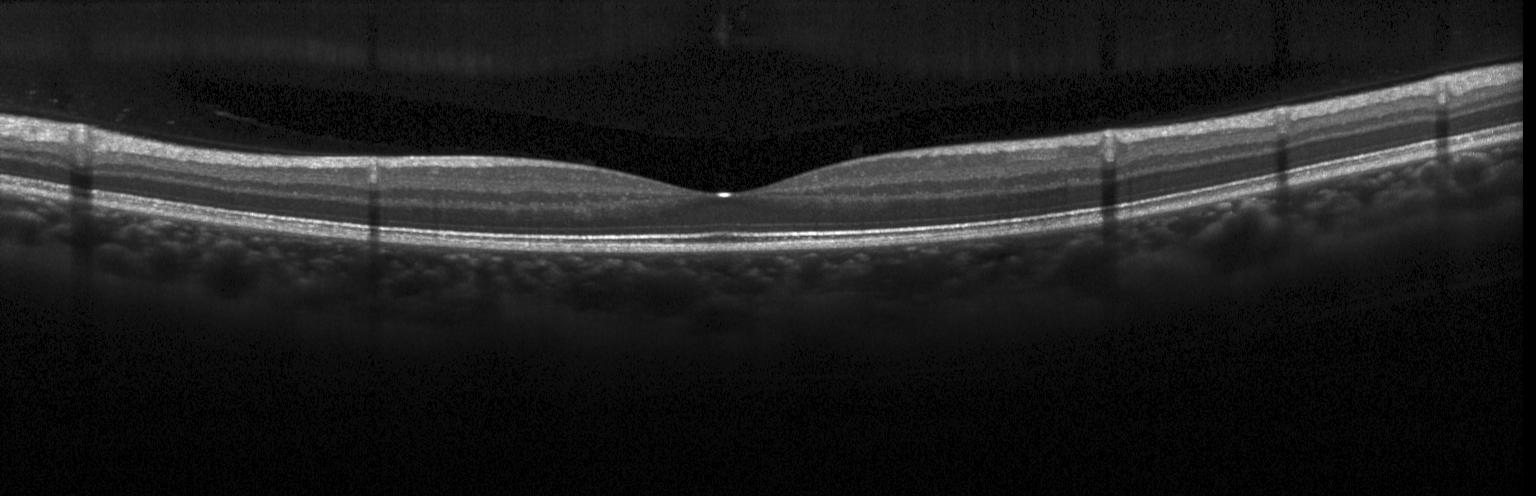

Neither choroidal neovascularization, diabetic macular edema, nor drusen.